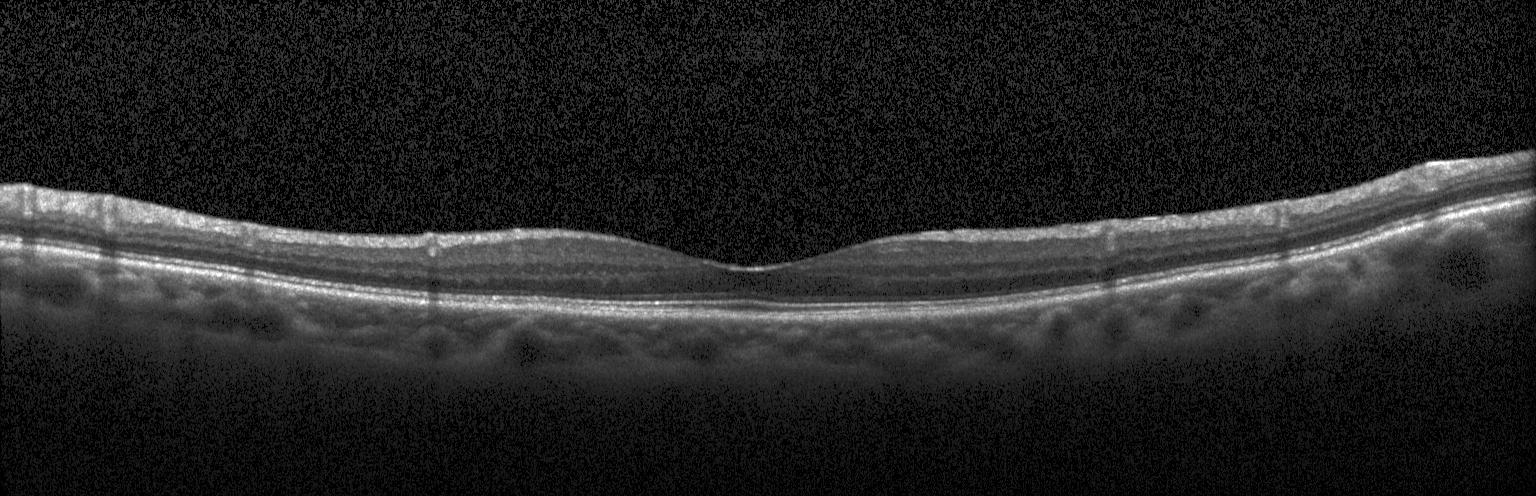
Heidelberg Spectralis. Retinal OCT B-scan.
Finding: no choroidal neovascularization, no diabetic macular edema, and no drusen.